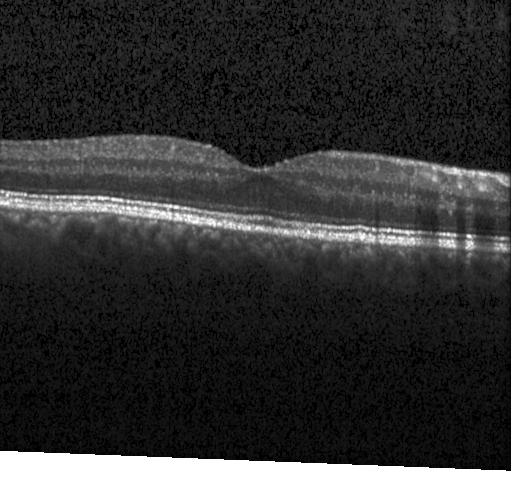
Optical coherence tomography scan, Heidelberg Spectralis, fovea-centered
No evidence of CNV, DME, or drusen.